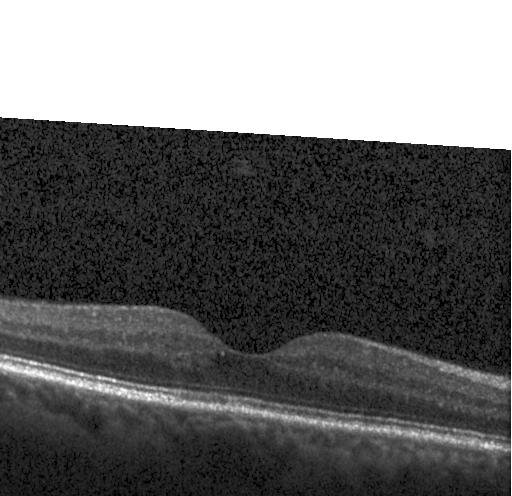 Heidelberg Spectralis · OCT B-scan · macular scan · spectral-domain OCT.
The scan shows neither CNV, DME, nor drusen.